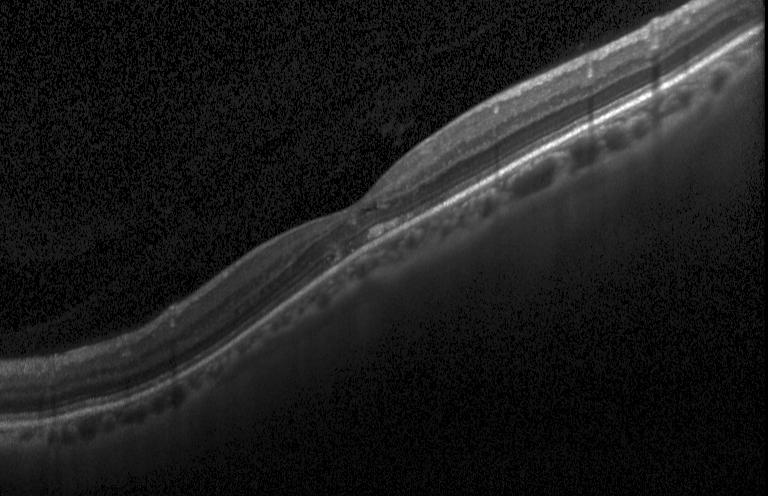
Impression: DME.